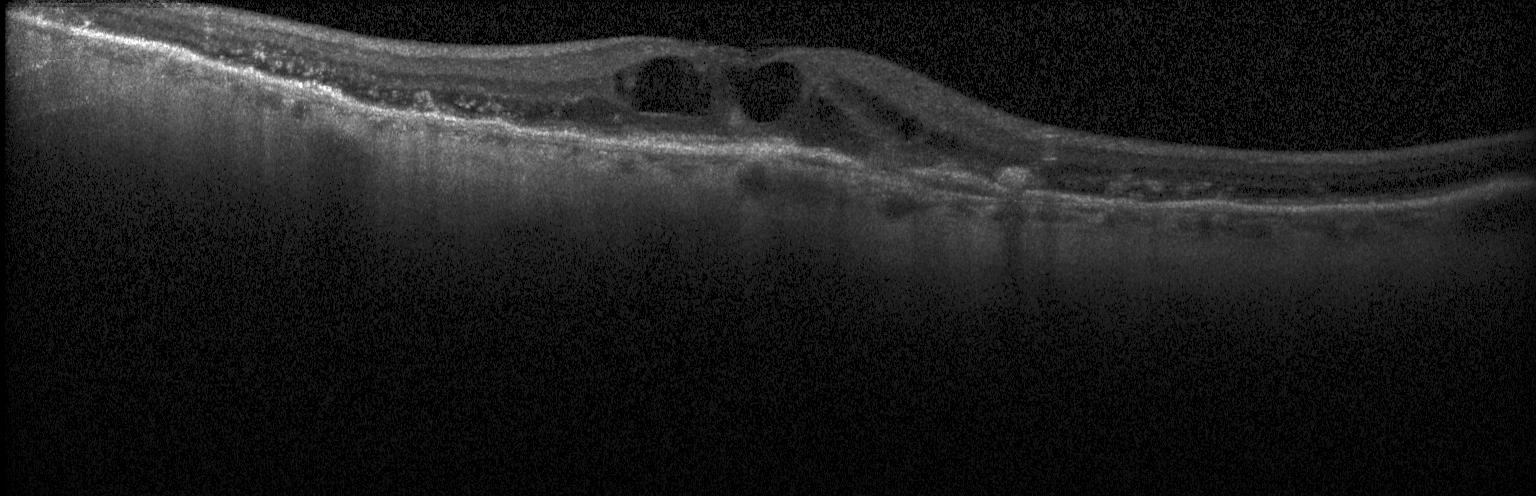 Finding: choroidal neovascularization (CNV).